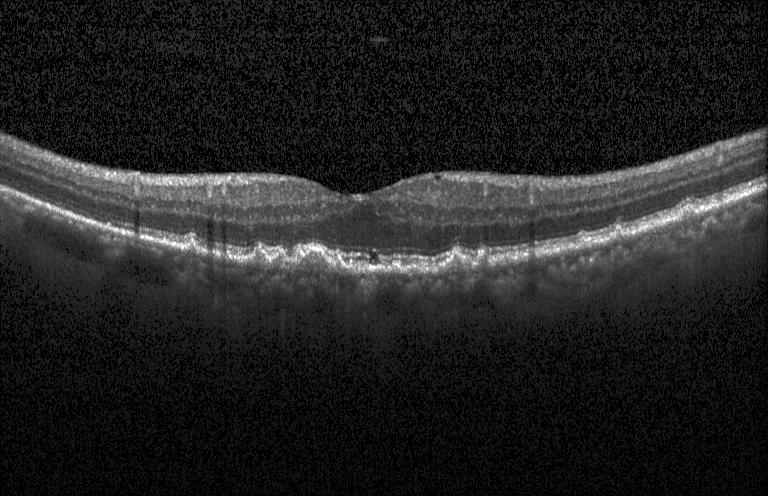 Retinal OCT B-scan. Impression: sub-RPE drusenoid deposits.